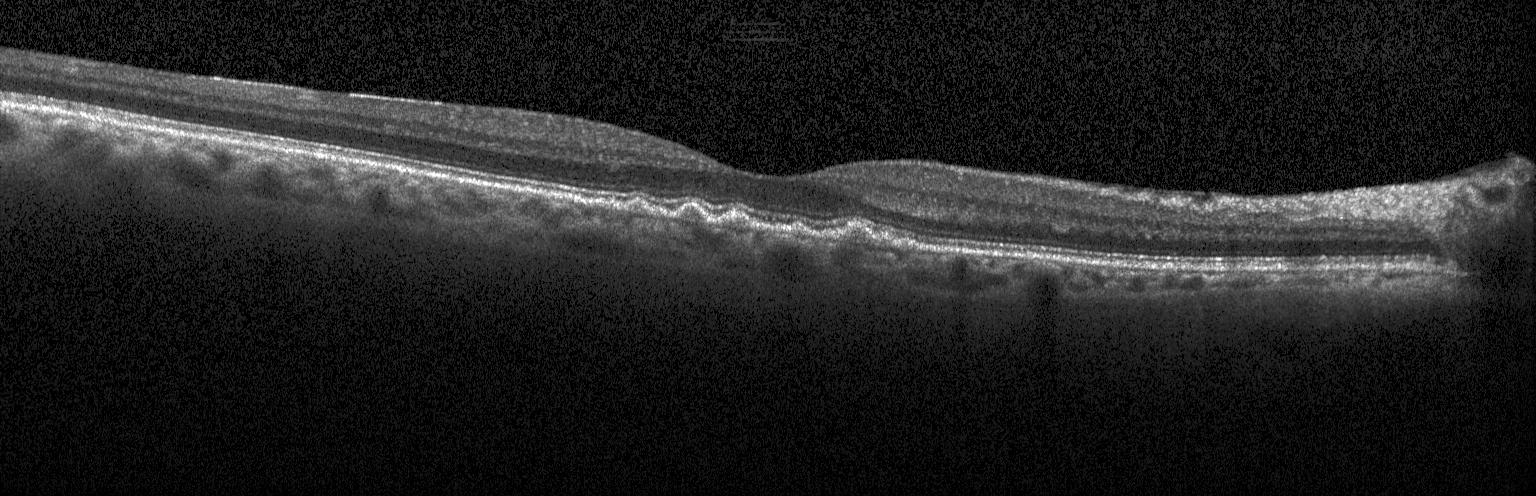
Retinal OCT B-scan. Through the macula — Diagnosis: sub-RPE drusenoid deposits.